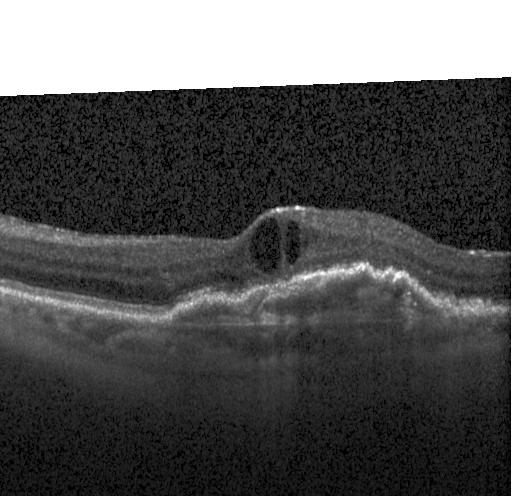

The scan shows choroidal neovascularization.